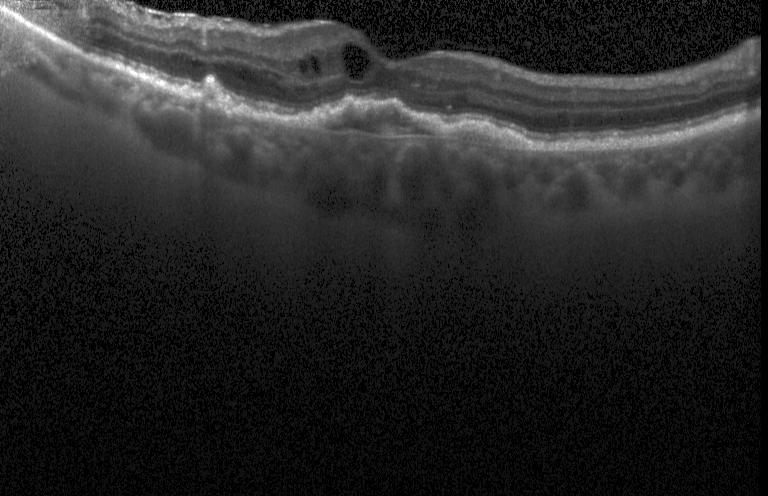 Heidelberg Spectralis, optical coherence tomography scan. This B-scan demonstrates choroidal neovascularization.